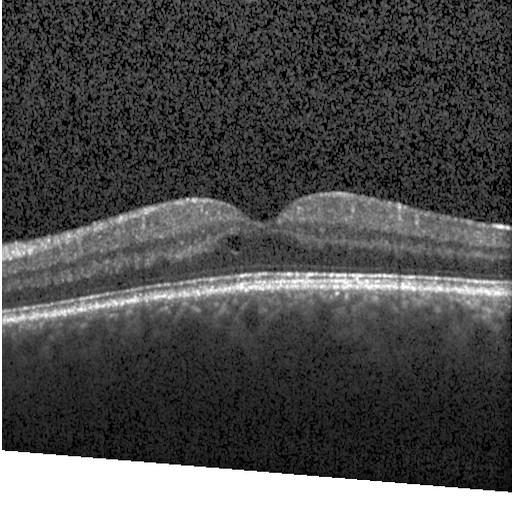 SD-OCT · retinal OCT cross-section · Heidelberg Spectralis OCT system.
Impression: diabetic macular edema (DME).